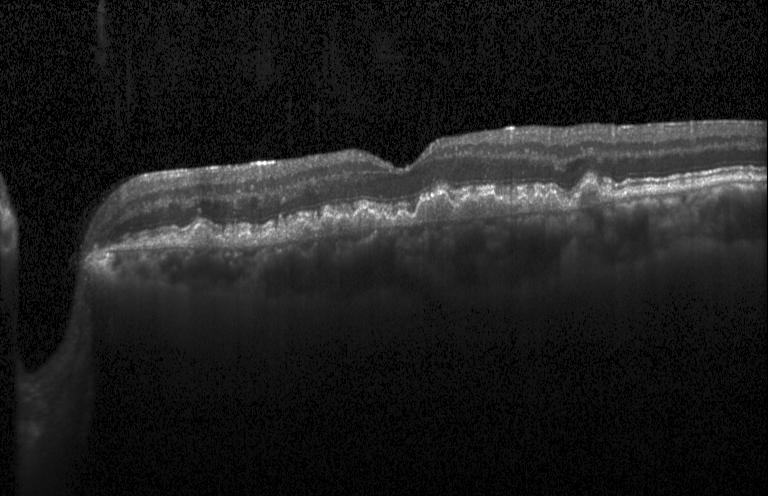
Finding: a choroidal neovascular membrane.